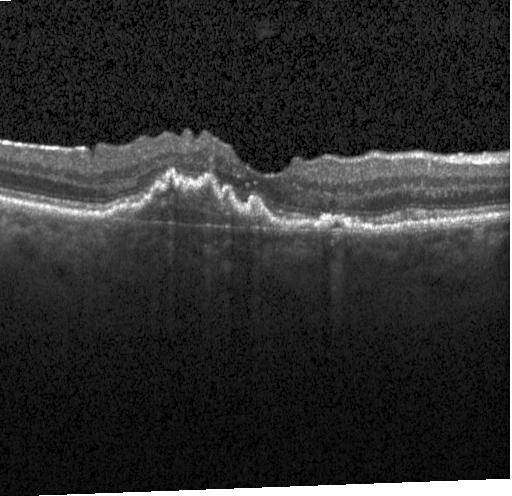 Retinal OCT cross-section showing a choroidal neovascular membrane.